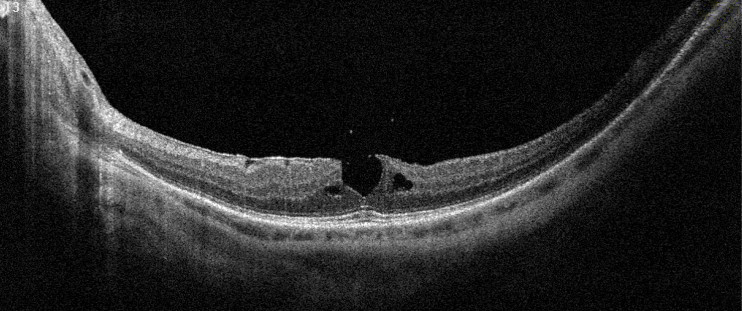
Retinal OCT cross-section showing vitreomacular interface disease (VID).